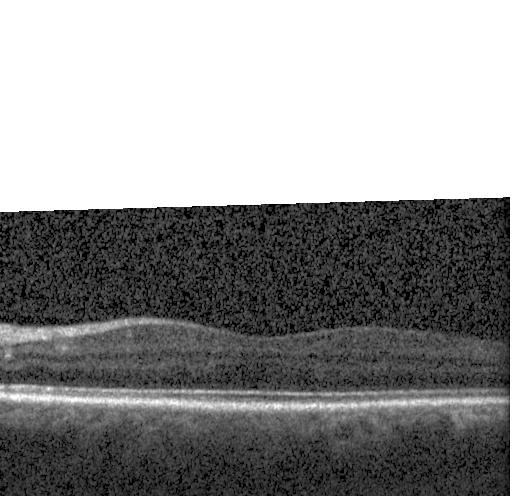 Finding: no choroidal neovascularization, diabetic macular edema, or drusen.